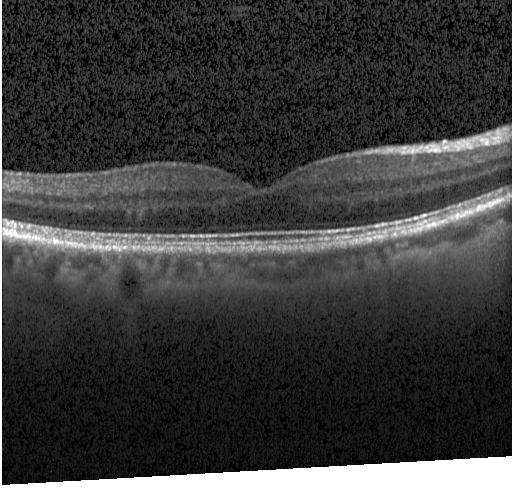 No evidence of choroidal neovascularization, diabetic macular edema, or drusen.